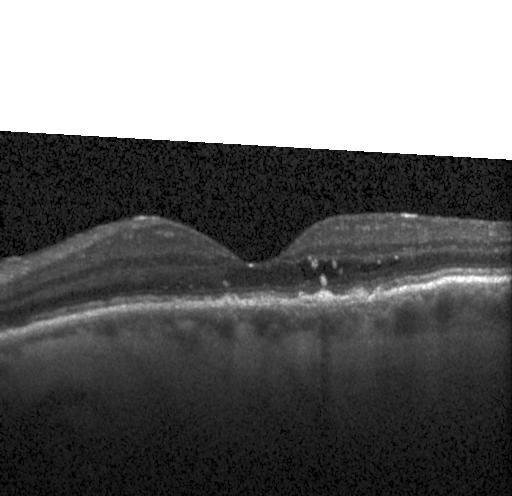 OCT line scan. Assessment: choroidal neovascularization (CNV).